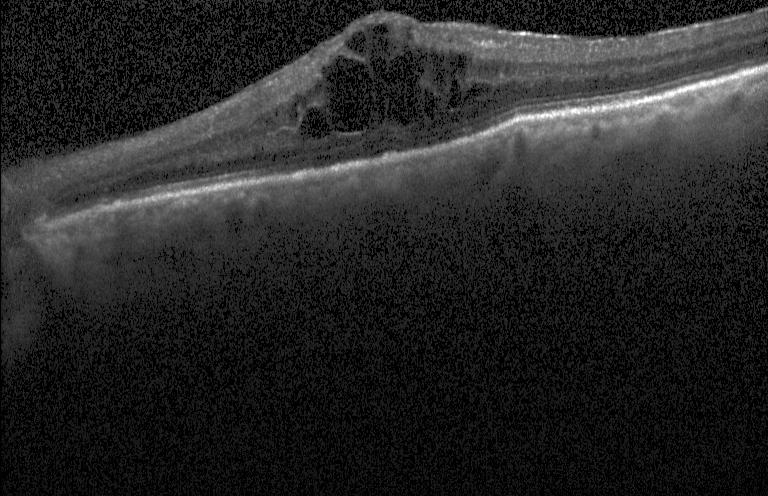 OCT line scan, Heidelberg Spectralis, spectral-domain OCT. Finding: DME.